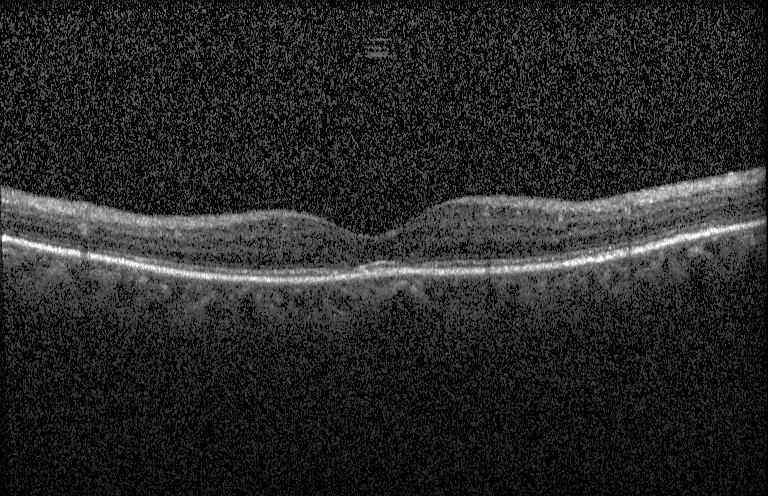 Fovea-centered. Heidelberg Spectralis OCT system. Retinal OCT B-scan.
Finding: neither CNV, DME, nor drusen.